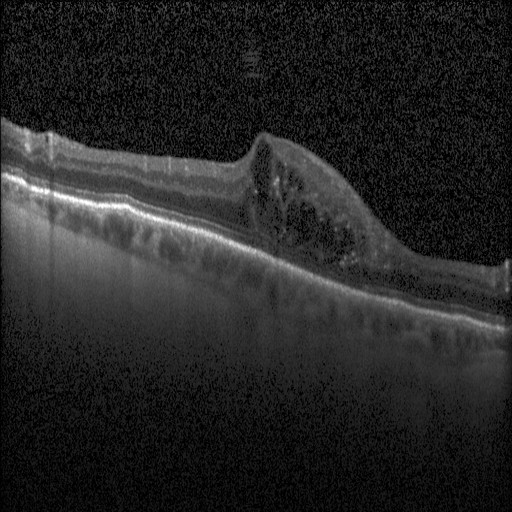
Spectral-domain optical coherence tomography. Instrument: Heidelberg Spectralis. Horizontal scan through the fovea. Retinal OCT cross-section
Dx: DME.